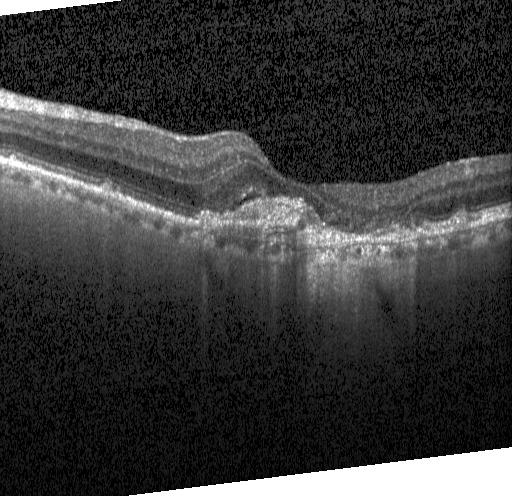 Optical coherence tomography scan · spectral-domain OCT.
CNV.